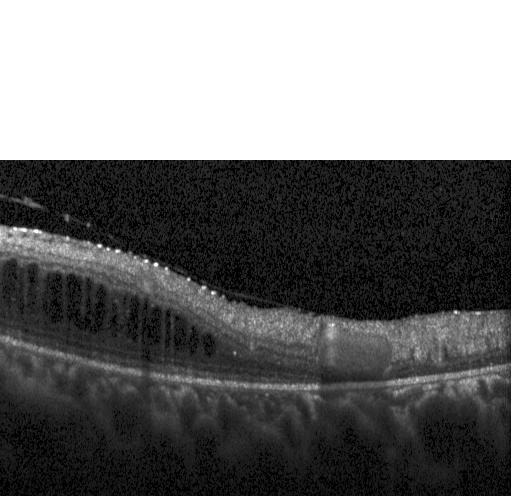 Impression: diabetic macular edema.